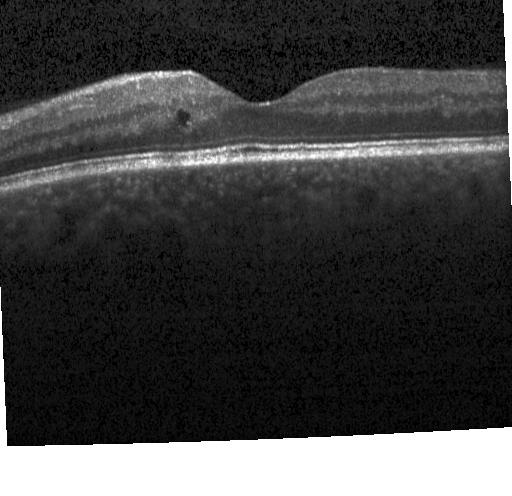

Through the macula. Heidelberg Spectralis OCT system. SD-OCT. OCT line scan. Assessment: DME.